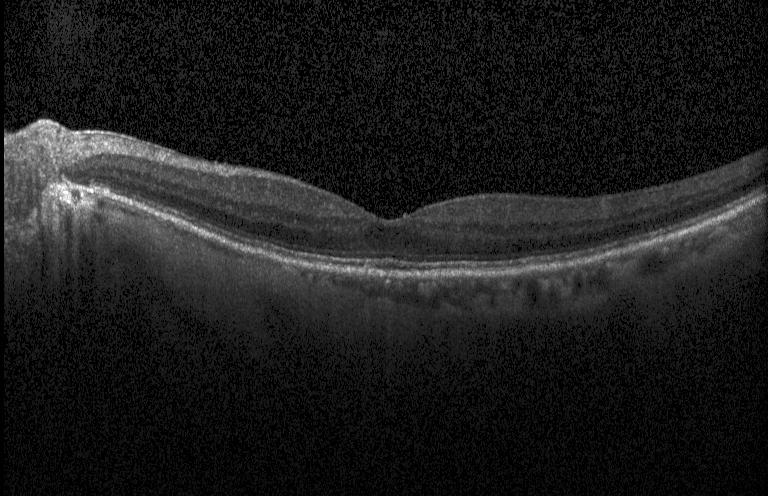 Macular OCT demonstrating no CNV, no DME, and no drusen.